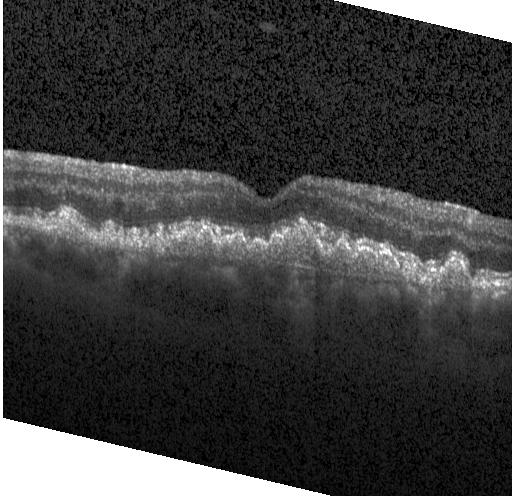
Optical coherence tomography B-scan. SD-OCT. Acquired on a Heidelberg Spectralis. Horizontal scan through the fovea.
OCT finding: CNV.